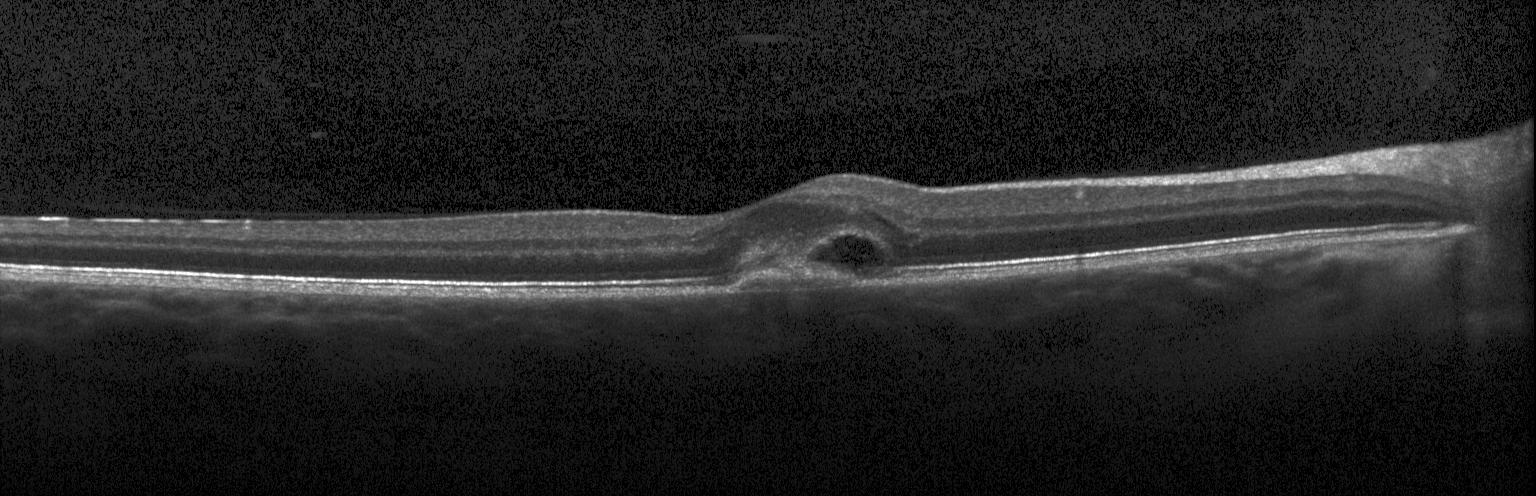 This B-scan demonstrates a choroidal neovascular membrane.